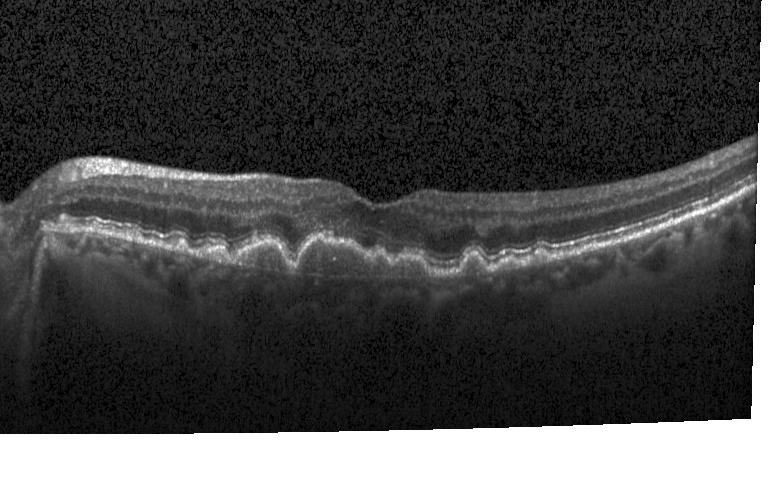

OCT B-scan. Spectral-domain optical coherence tomography. Instrument: Heidelberg Spectralis. Macular OCT: a choroidal neovascular membrane.